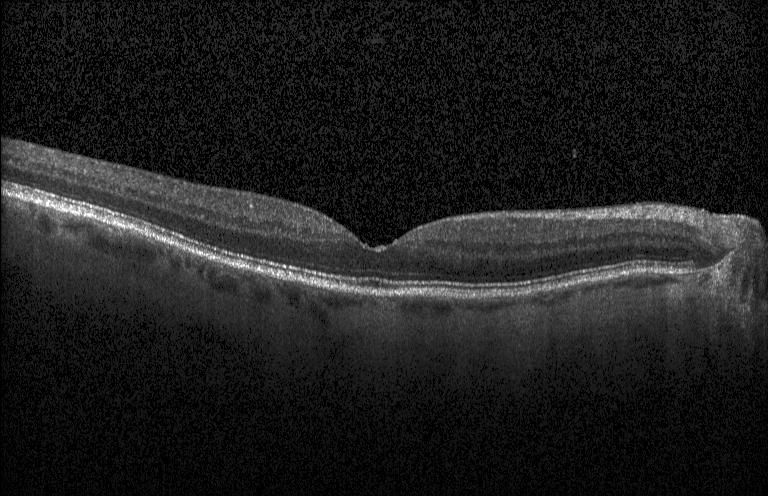
OCT B-scan, centered on the fovea, Heidelberg Spectralis — Macular OCT: no CNV, no DME, and no drusen.